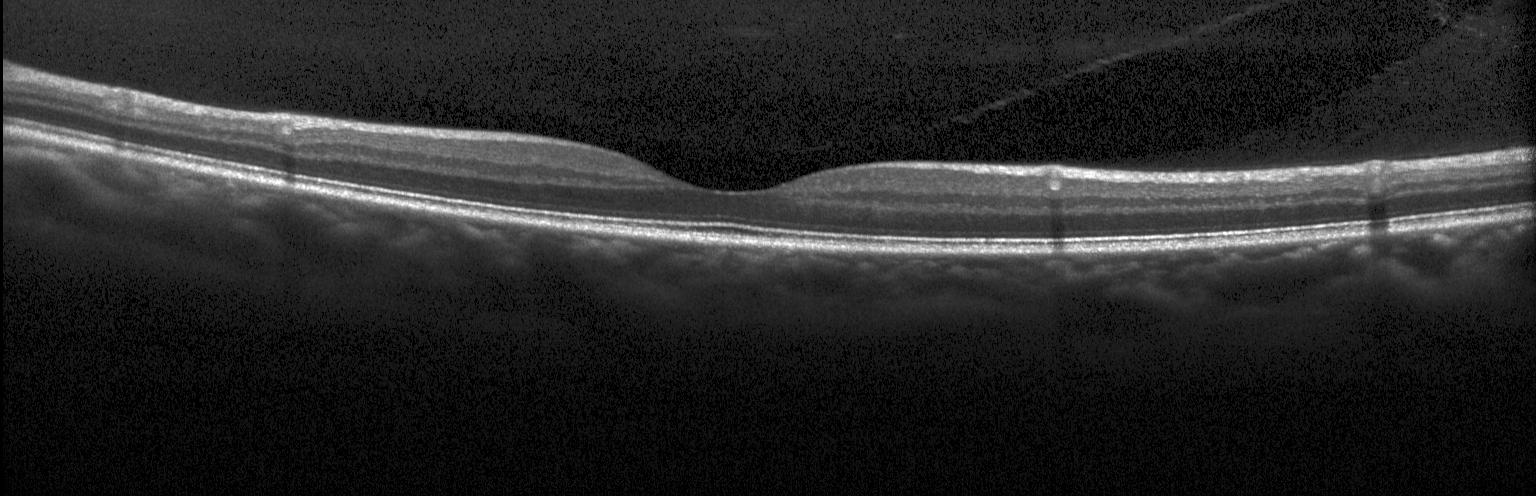 Diagnosis: no CNV, DME, or drusen.